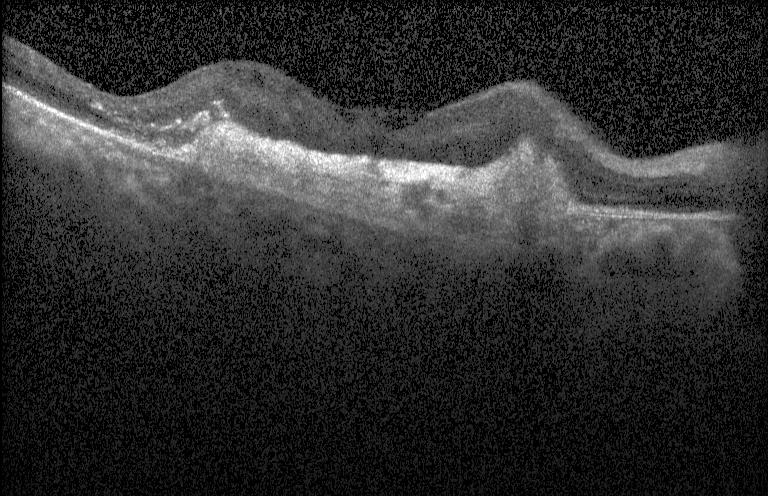

Retinal OCT cross-section. Heidelberg Spectralis OCT system. Macular scan. Spectral-domain optical coherence tomography. A choroidal neovascular membrane.